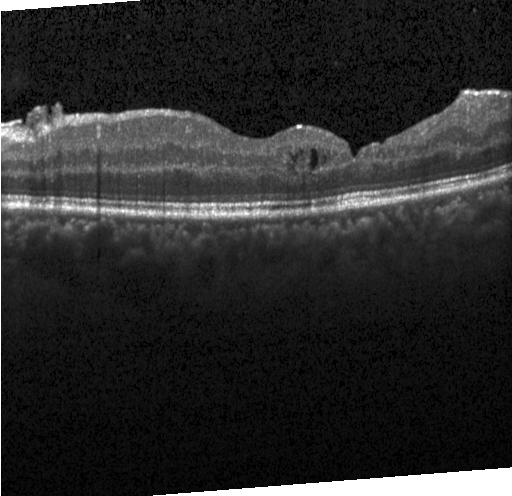

Impression: diabetic macular edema (DME).